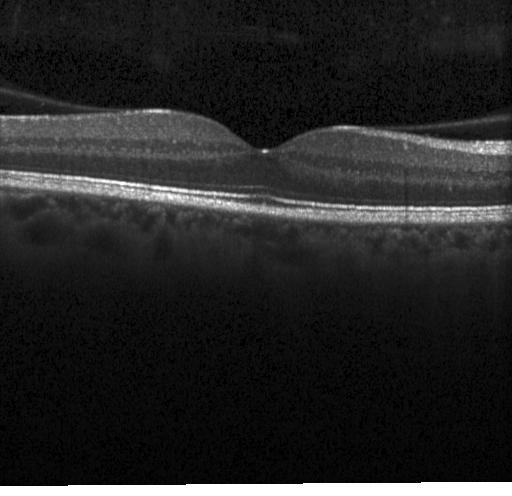
Spectral-domain OCT · centered on the fovea · optical coherence tomography B-scan. Impression: no choroidal neovascularization, diabetic macular edema, or drusen.